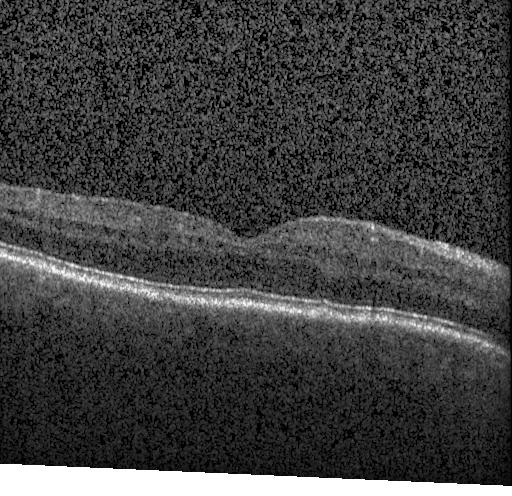 Optical coherence tomography B-scan, Heidelberg Spectralis OCT system, macular scan
Finding: neither choroidal neovascularization, diabetic macular edema, nor drusen.